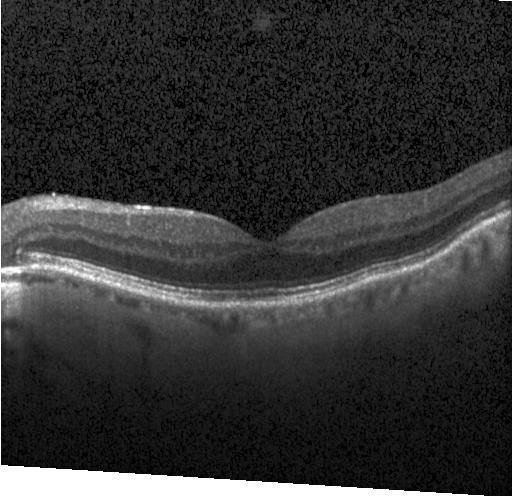 Finding: no evidence of choroidal neovascularization, diabetic macular edema, or drusen.